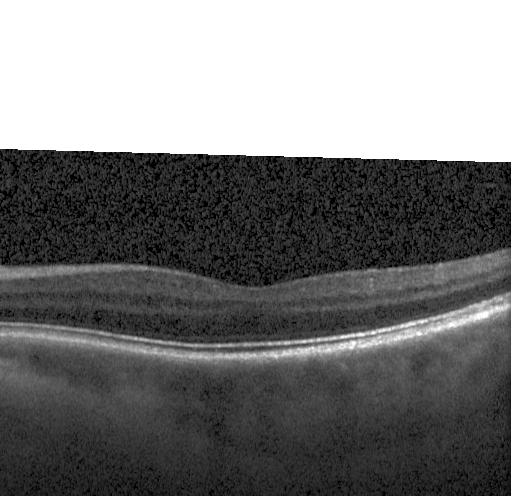

SD-OCT. Through the macula. OCT line scan.
OCT finding: no choroidal neovascularization, no diabetic macular edema, and no drusen.